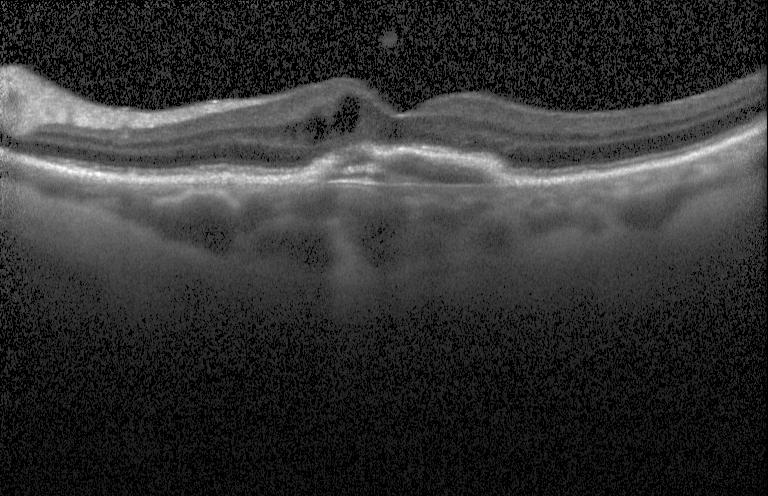 Instrument: Heidelberg Spectralis, optical coherence tomography scan, through the macula — Impression: choroidal neovascularization.